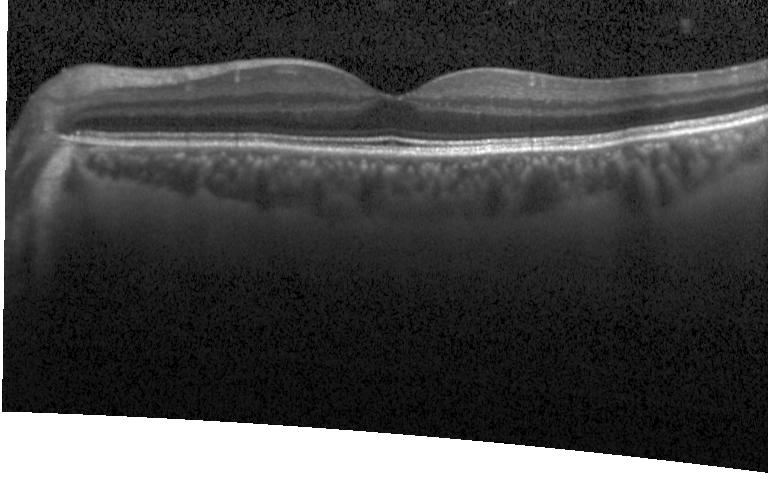
Heidelberg Spectralis, spectral-domain OCT, OCT B-scan, fovea-centered — Neither choroidal neovascularization, diabetic macular edema, nor drusen.